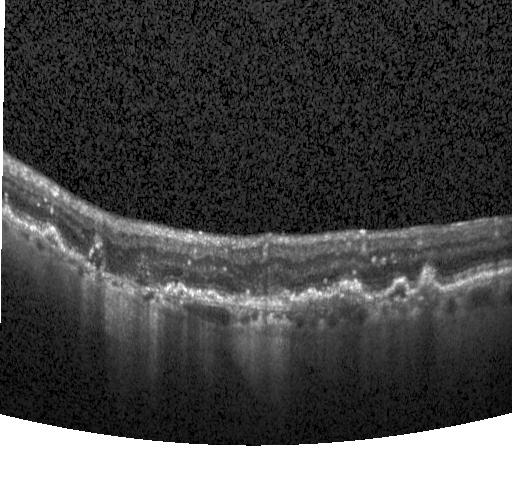

Finding: a choroidal neovascular membrane.